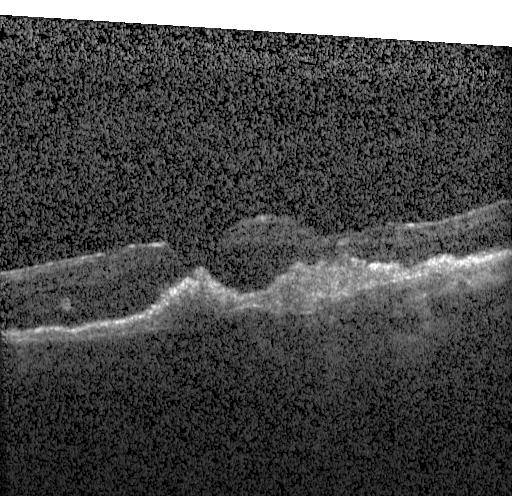
Finding: a choroidal neovascular membrane.